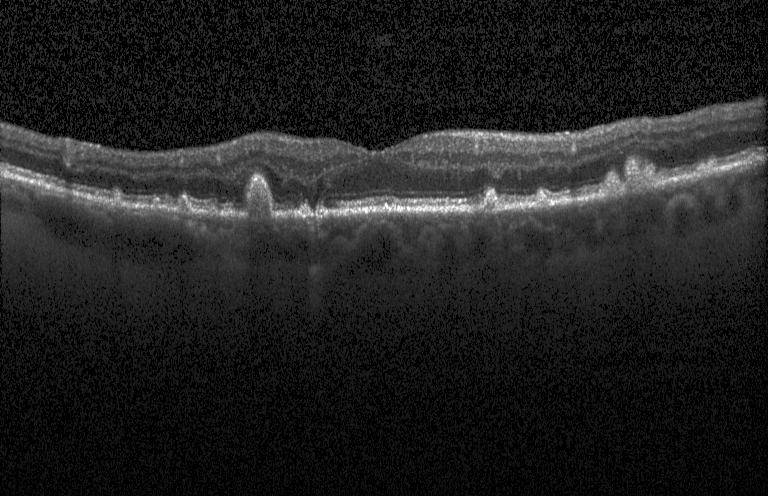 Optical coherence tomography scan. This B-scan demonstrates sub-RPE drusenoid deposits.